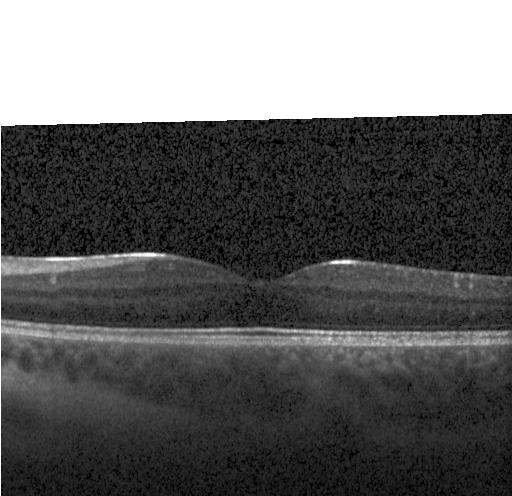

Diagnosis: no choroidal neovascularization, no diabetic macular edema, and no drusen.